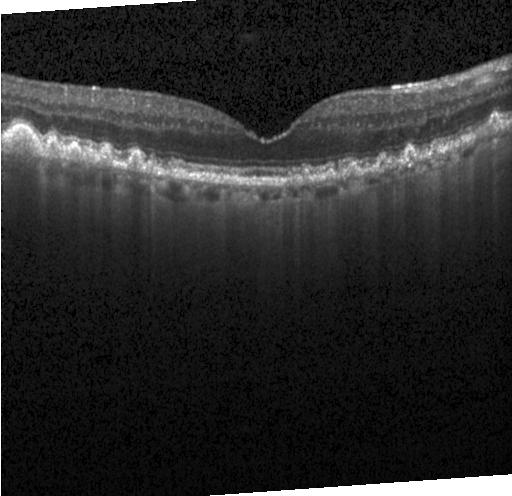
Heidelberg Spectralis OCT system; OCT line scan; macular scan.
Diagnosis: multiple drusen.